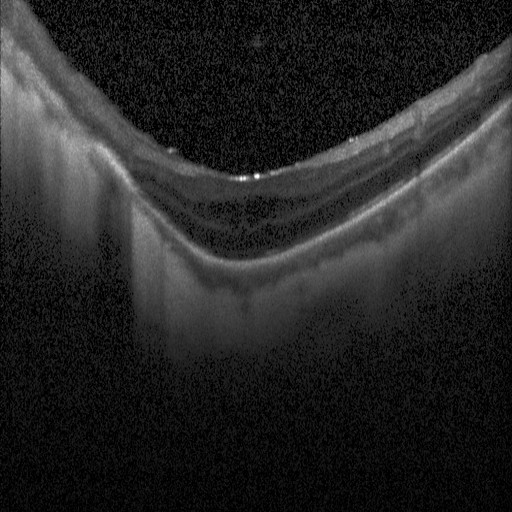
Optical coherence tomography scan.
Impression: diabetic macular edema.